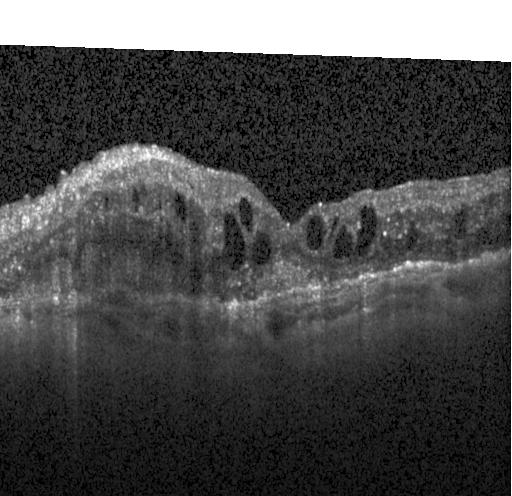

OCT line scan; spectral-domain OCT; fovea-centered; acquired on a Heidelberg Spectralis
Finding: a choroidal neovascular membrane.